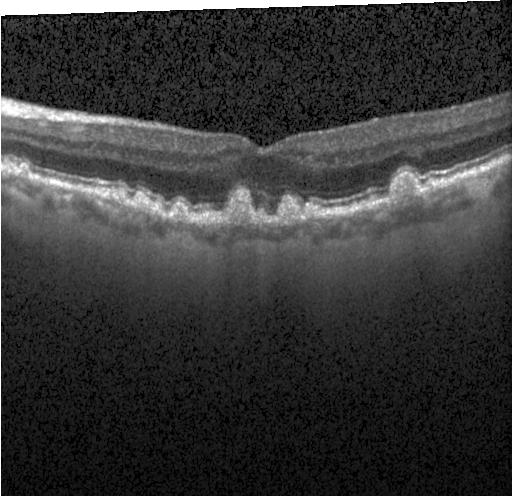 SD-OCT. Through the macula. Retinal OCT cross-section. Heidelberg Spectralis. Diagnosis: drusen.